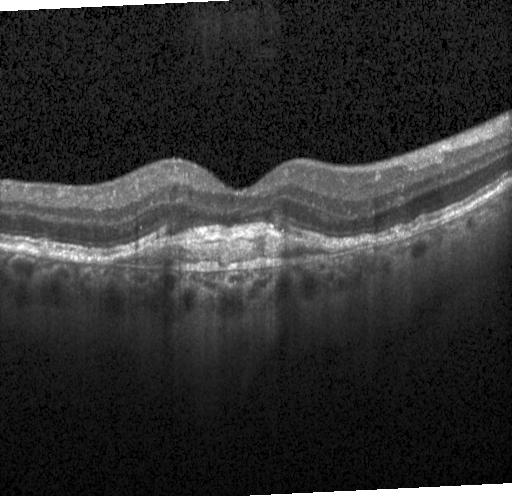
Impression: a choroidal neovascular membrane.